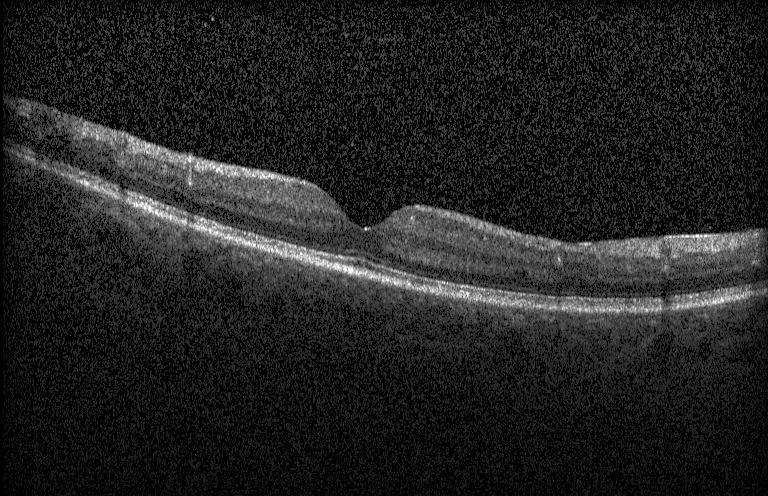 OCT B-scan, spectral-domain optical coherence tomography, fovea-centered, instrument: Heidelberg Spectralis. Diagnosis: no CNV, no DME, and no drusen.